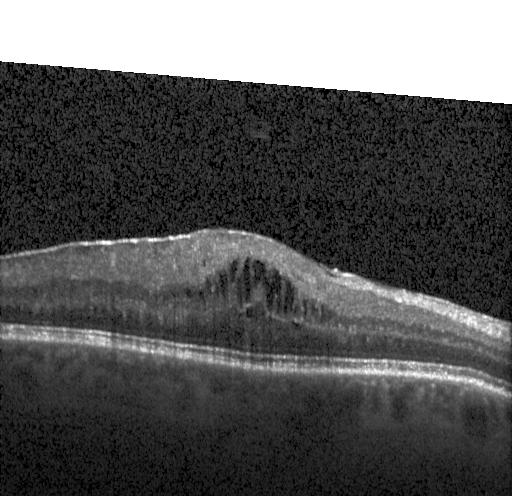
Optical coherence tomography scan, acquired on a Heidelberg Spectralis. Assessment: diabetic macular edema.